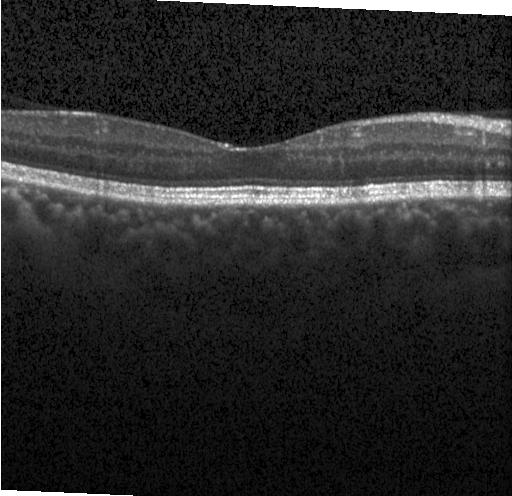
Spectral-domain optical coherence tomography · centered on the fovea · Heidelberg Spectralis · optical coherence tomography B-scan. Finding: no choroidal neovascularization, diabetic macular edema, or drusen.